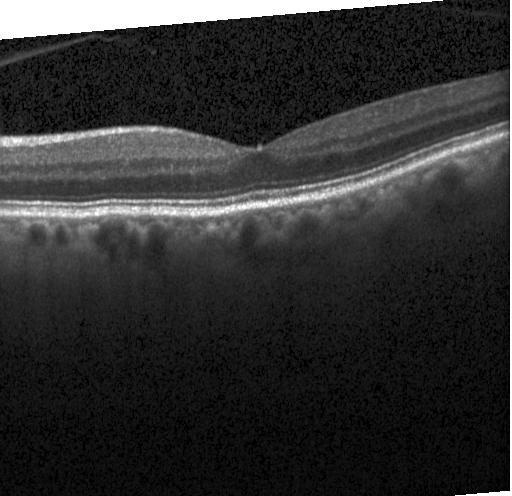
Optical coherence tomography B-scan · Heidelberg Spectralis OCT system.
Impression: no choroidal neovascularization, diabetic macular edema, or drusen.